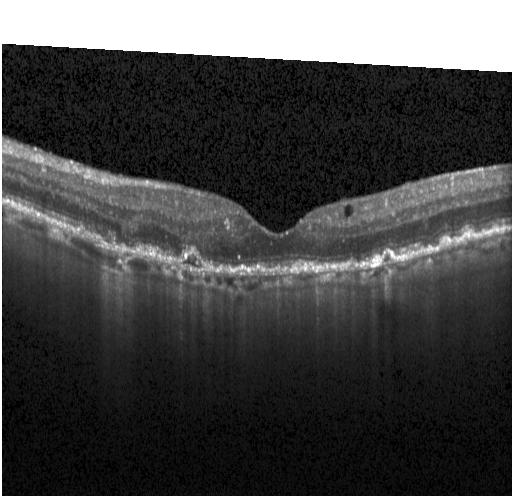

Assessment: a choroidal neovascular membrane.